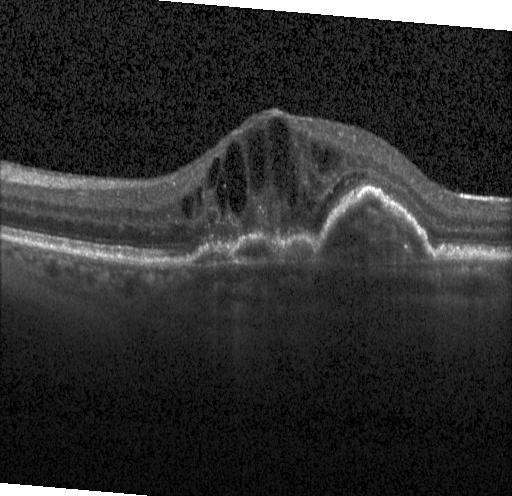 Finding: a choroidal neovascular membrane.